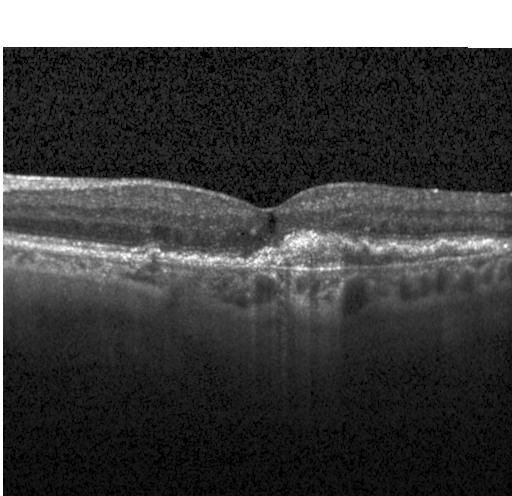
Retinal OCT cross-section
Dx: a choroidal neovascular membrane.